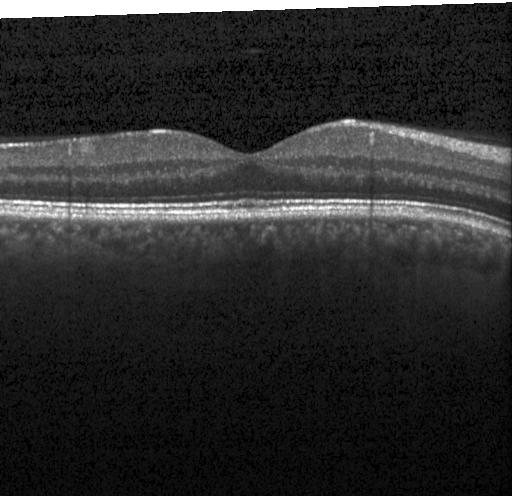
Impression: no evidence of choroidal neovascularization, diabetic macular edema, or drusen.